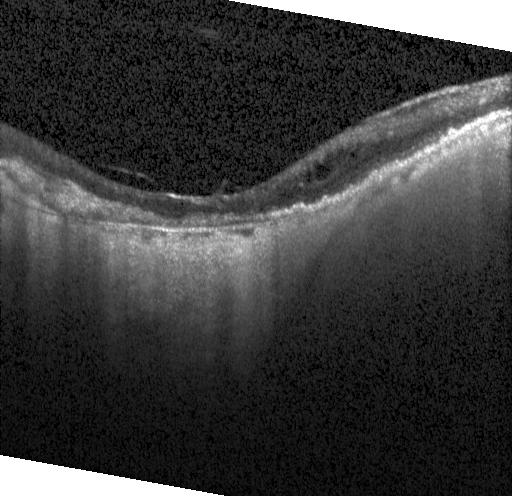 Retinal OCT cross-section — This B-scan demonstrates a choroidal neovascular membrane.